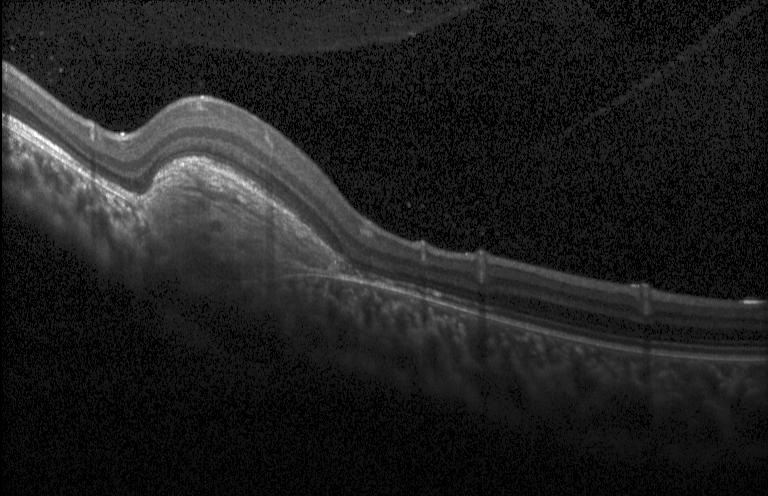

Macular OCT: CNV.